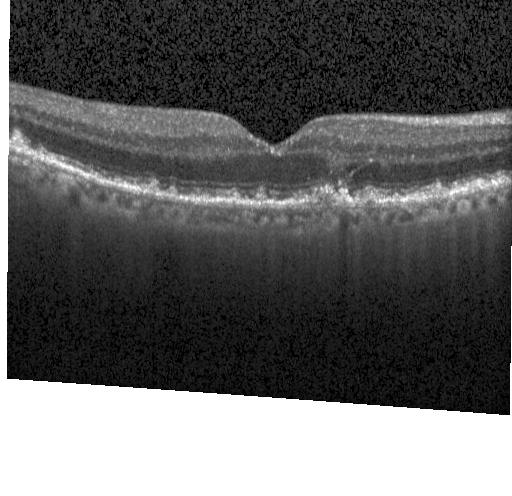

Spectral-domain optical coherence tomography; OCT line scan.
Sub-RPE drusenoid deposits.